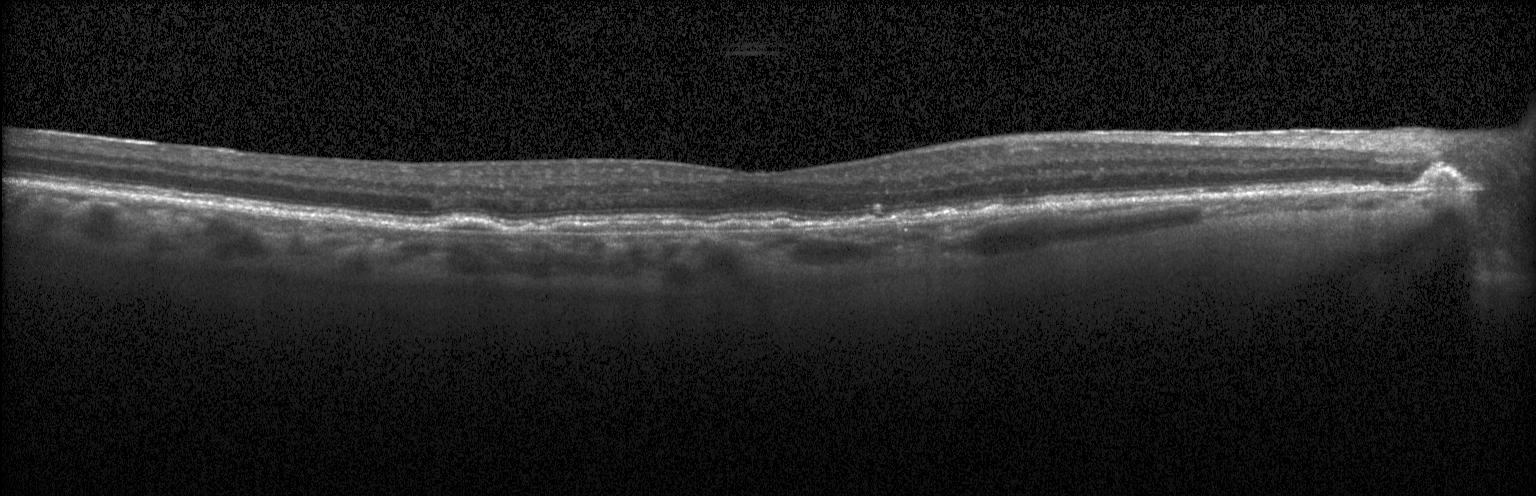
Through the macula · retinal OCT cross-section · spectral-domain optical coherence tomography · Heidelberg Spectralis OCT system
Macular OCT: choroidal neovascularization.